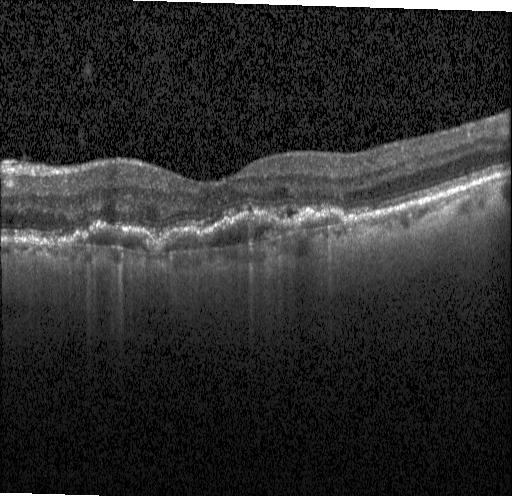

OCT line scan. Acquired on a Heidelberg Spectralis.
Assessment: a choroidal neovascular membrane.